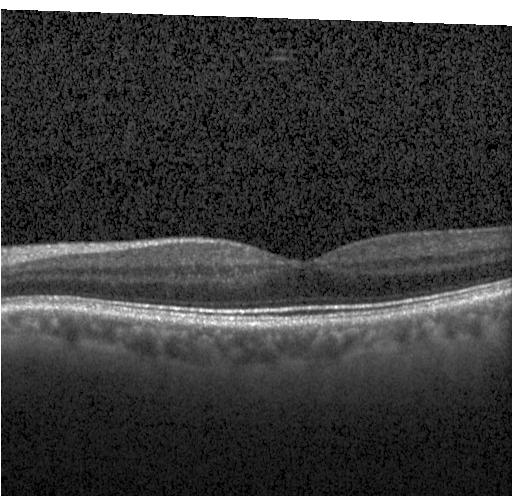 This B-scan demonstrates neither choroidal neovascularization, diabetic macular edema, nor drusen.